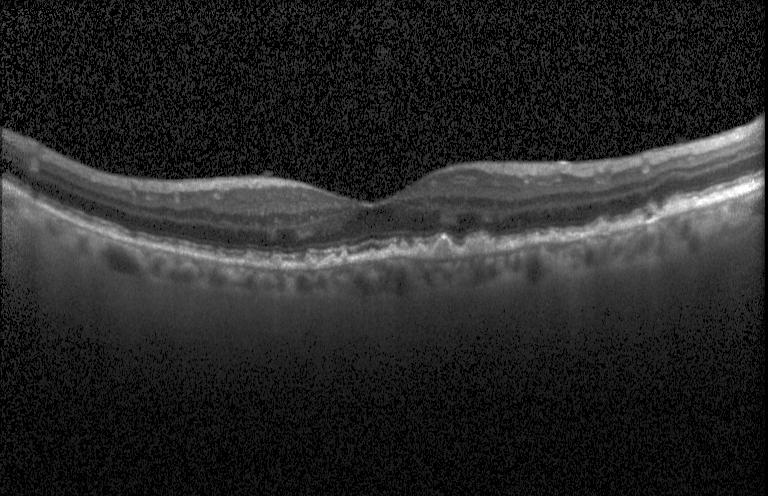
OCT B-scan.
Multiple drusen.